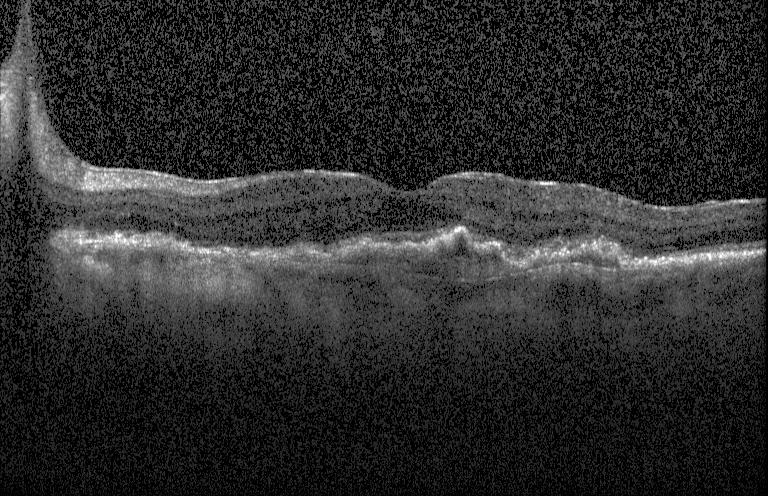 Optical coherence tomography B-scan — Assessment: CNV.